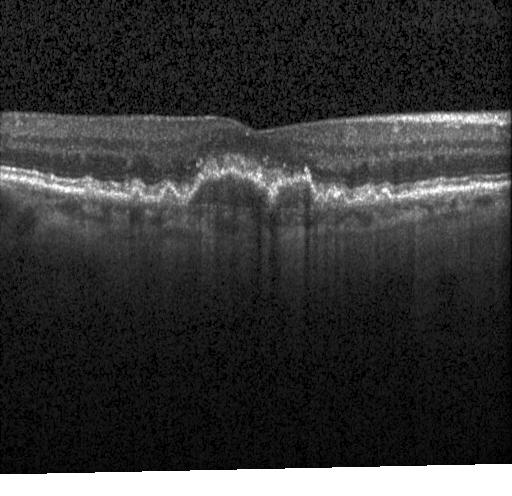

Optical coherence tomography B-scan.
Finding: CNV.